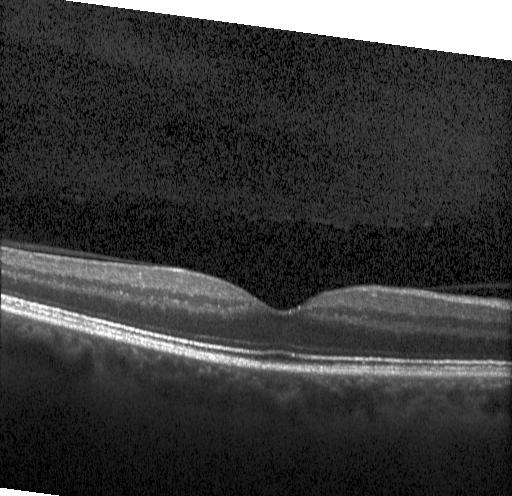
Optical coherence tomography scan. SD-OCT. Fovea-centered. Heidelberg Spectralis.
No CNV, DME, or drusen.